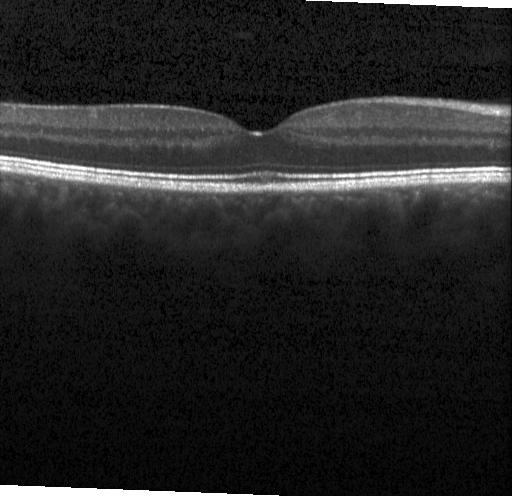
Centered on the fovea. OCT line scan. Finding: no choroidal neovascularization, diabetic macular edema, or drusen.